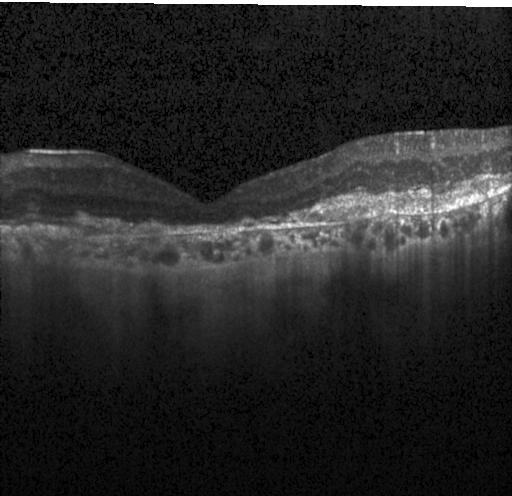
Fovea-centered, retinal OCT B-scan.
Impression: a choroidal neovascular membrane.